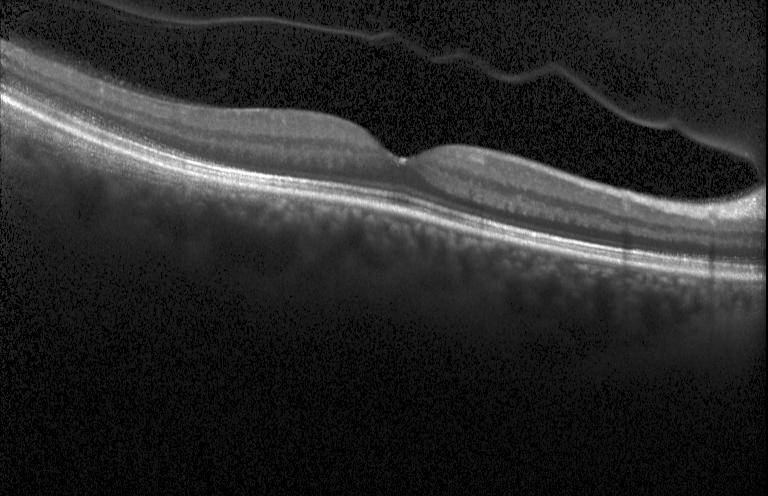
Acquired on a Heidelberg Spectralis, retinal OCT B-scan, SD-OCT, centered on the fovea. This B-scan demonstrates neither choroidal neovascularization, diabetic macular edema, nor drusen.